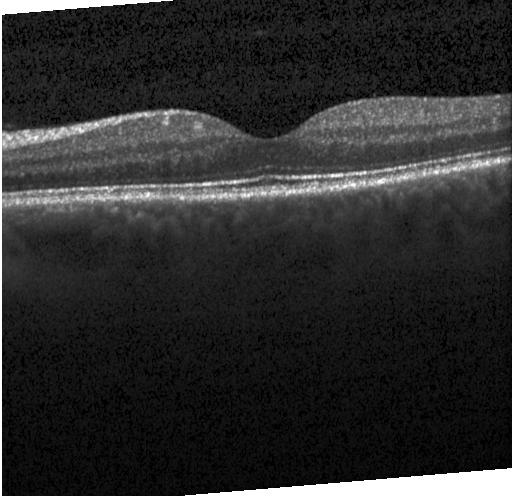 Spectral-domain optical coherence tomography · fovea-centered · optical coherence tomography B-scan · Heidelberg Spectralis OCT system — Dx: no CNV, DME, or drusen.